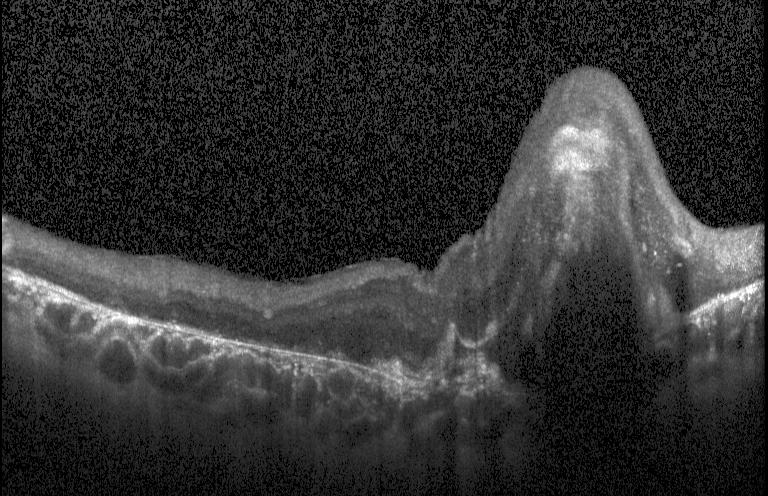

A choroidal neovascular membrane.